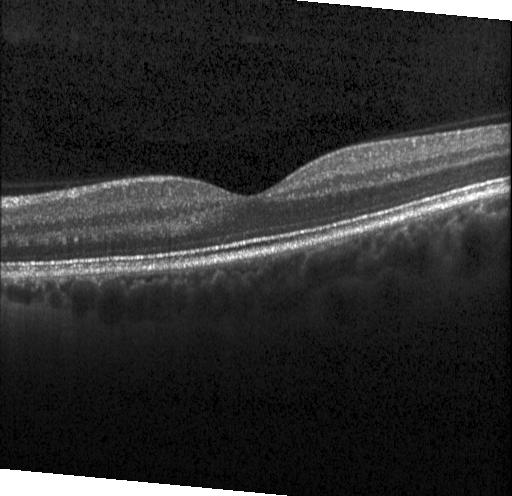 No choroidal neovascularization, diabetic macular edema, or drusen.